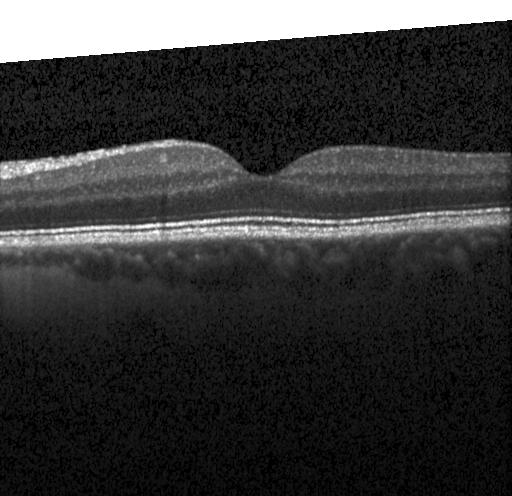 Retinal OCT B-scan. Horizontal scan through the fovea. SD-OCT. Heidelberg Spectralis OCT system. OCT finding: neither choroidal neovascularization, diabetic macular edema, nor drusen.